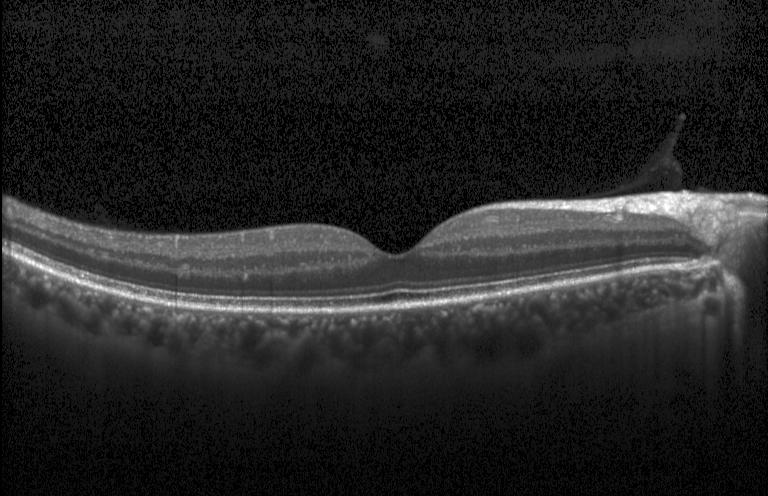
Macular OCT demonstrating no CNV, DME, or drusen.